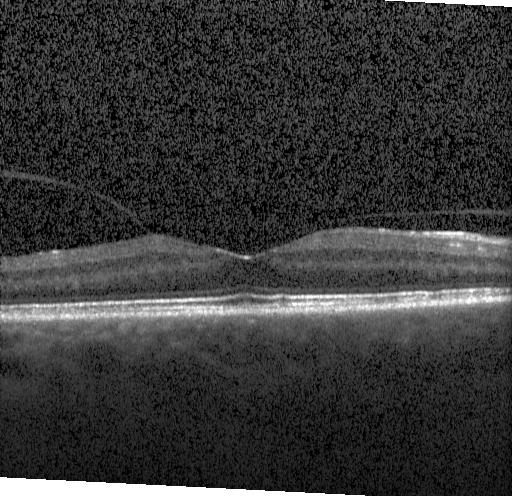
Dx: no choroidal neovascularization, no diabetic macular edema, and no drusen.